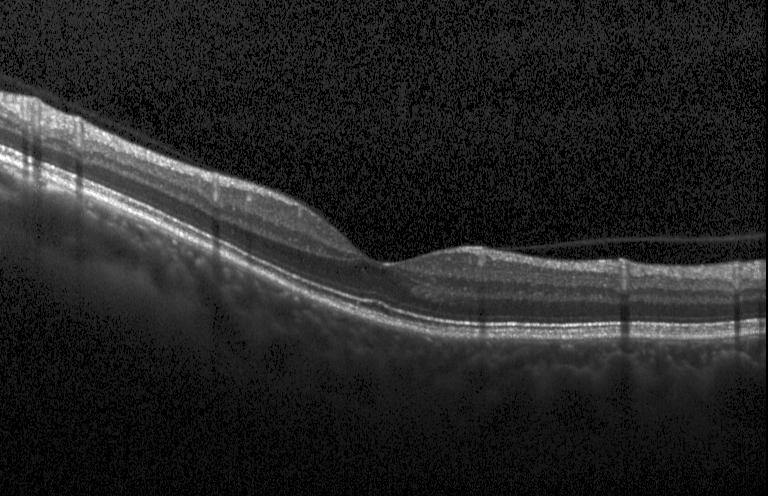

Retinal OCT cross-section showing no evidence of choroidal neovascularization, diabetic macular edema, or drusen.